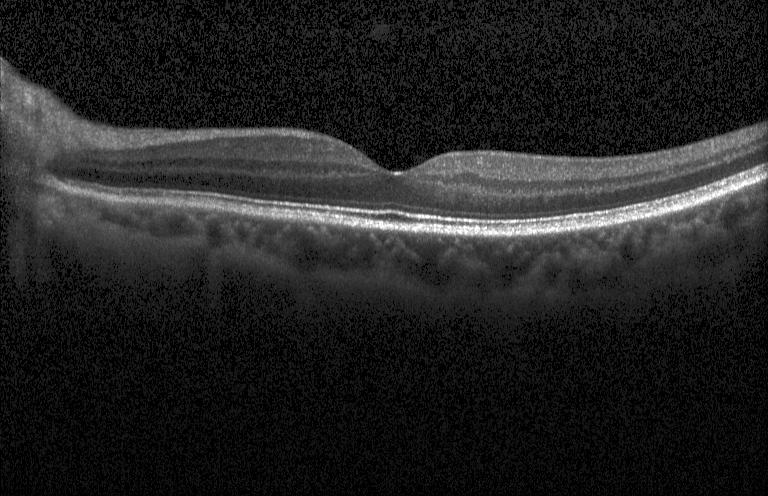 Impression: no CNV, no DME, and no drusen.